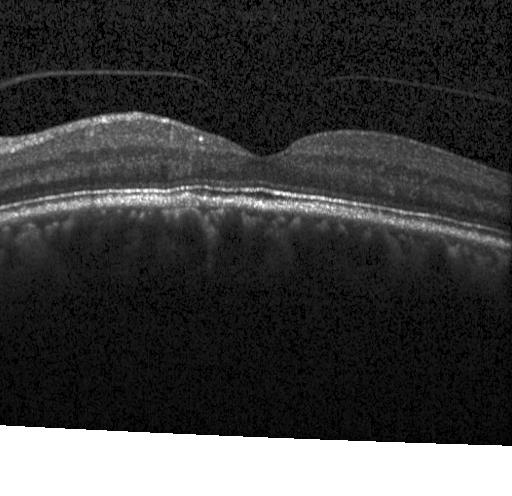

Impression: no choroidal neovascularization, diabetic macular edema, or drusen.